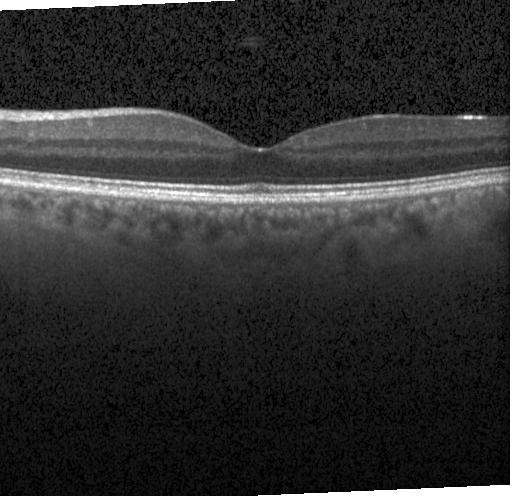
Spectral-domain OCT B-scan: no CNV, no DME, and no drusen.